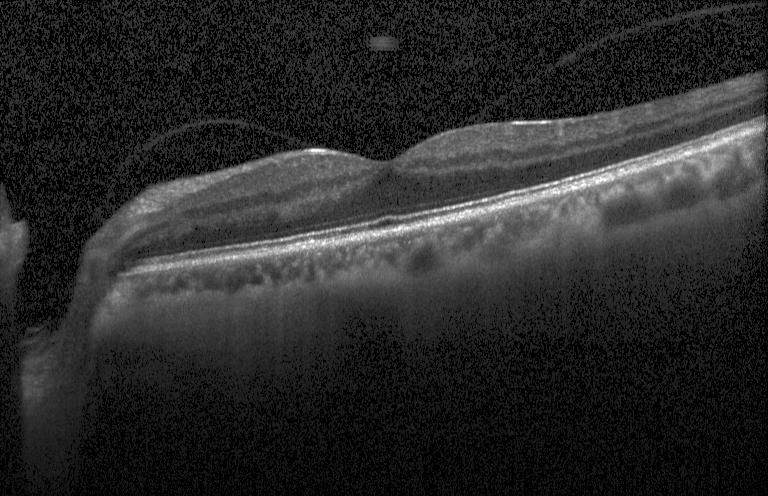 Macular OCT: no choroidal neovascularization, no diabetic macular edema, and no drusen.